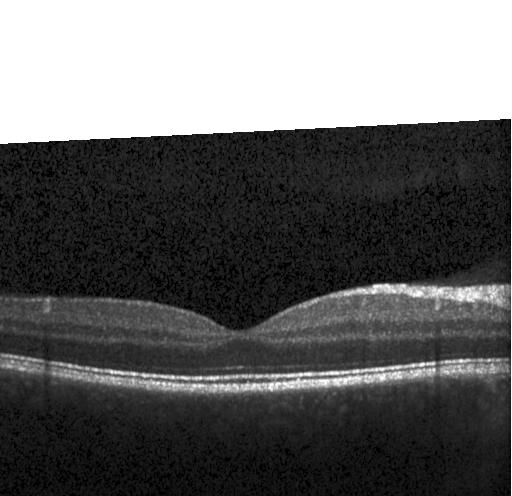

Spectral-domain optical coherence tomography; horizontal scan through the fovea; retinal OCT cross-section; Heidelberg Spectralis OCT system — This B-scan demonstrates no CNV, no DME, and no drusen.